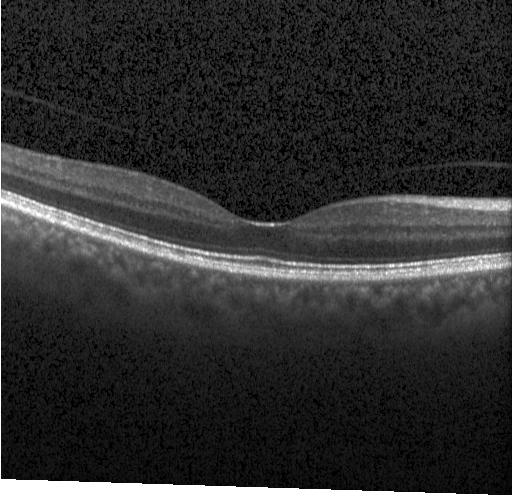 Spectral-domain OCT. OCT B-scan. Heidelberg Spectralis
Diagnosis: neither choroidal neovascularization, diabetic macular edema, nor drusen.